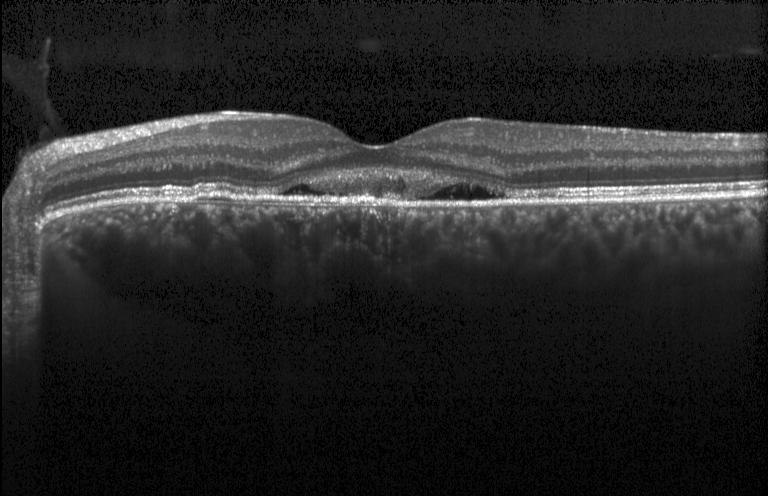 OCT B-scan — Macular OCT: a choroidal neovascular membrane.